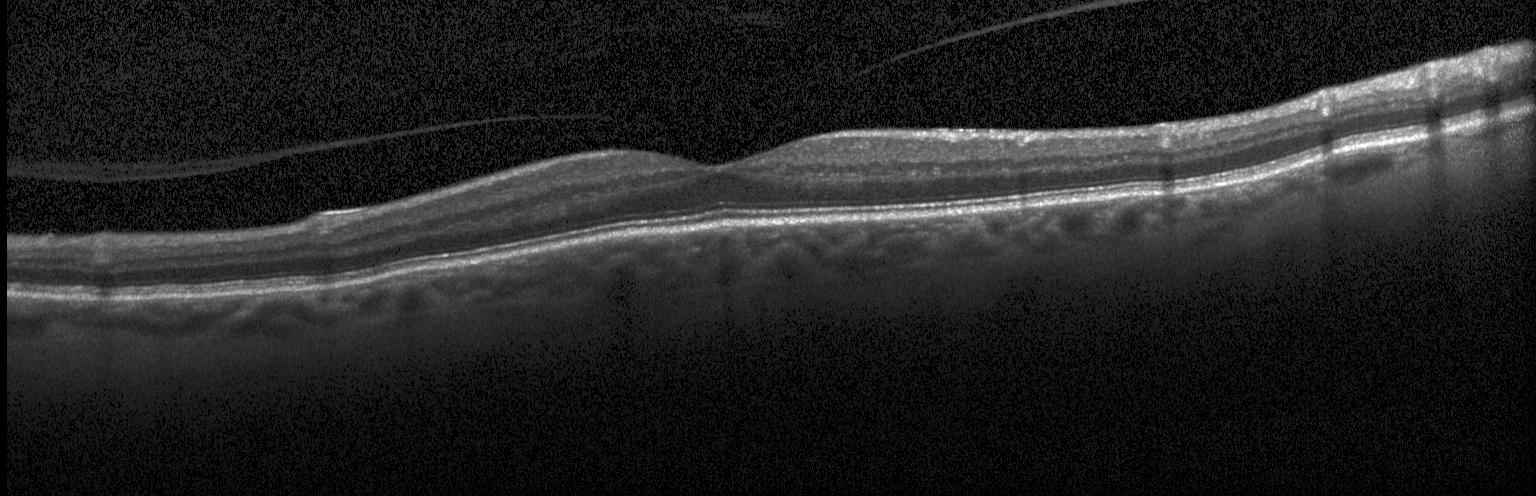

SD-OCT; acquired on a Heidelberg Spectralis; optical coherence tomography scan
The scan shows no CNV, no DME, and no drusen.